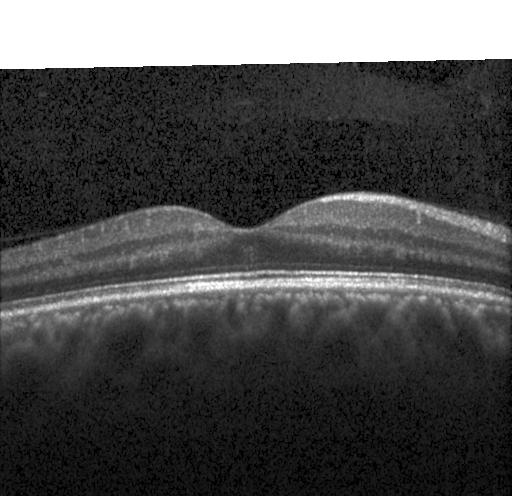

Optical coherence tomography B-scan. Spectral-domain OCT. Heidelberg Spectralis. Fovea-centered — Diagnosis: no evidence of choroidal neovascularization, diabetic macular edema, or drusen.